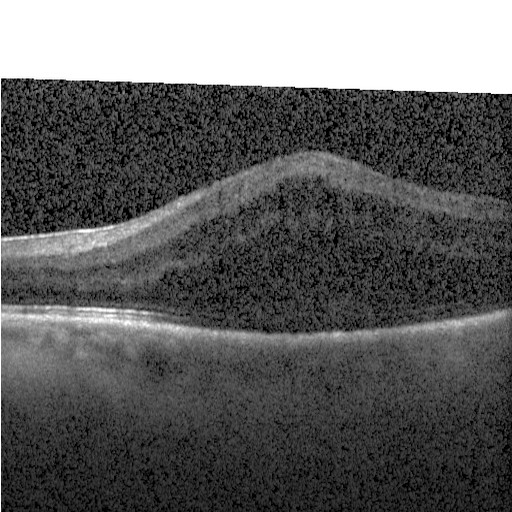
OCT B-scan; spectral-domain optical coherence tomography.
Finding: diabetic macular edema (DME).